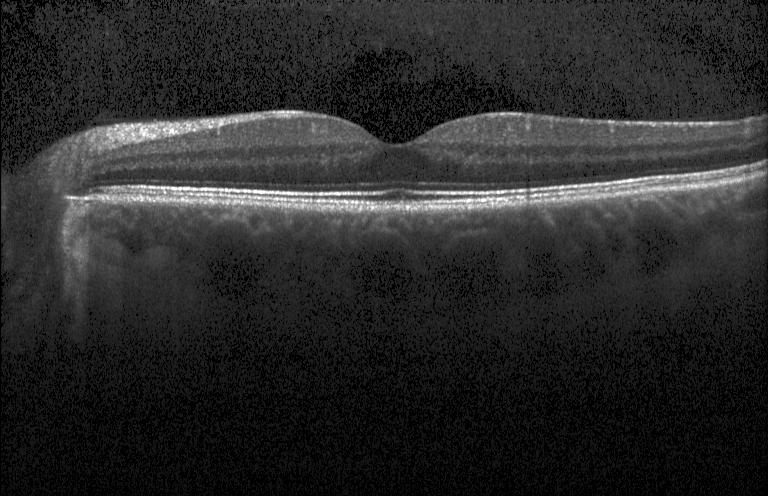

OCT scan showing no CNV, DME, or drusen.